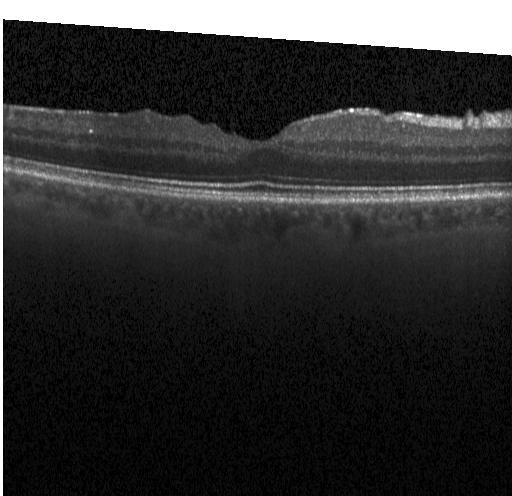
OCT finding: no CNV, DME, or drusen.